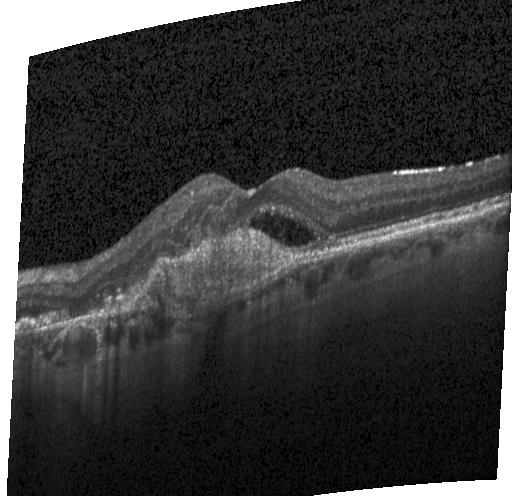 OCT finding: CNV.